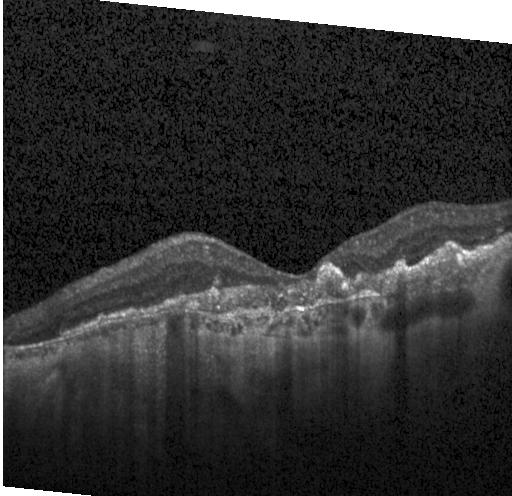
Finding: a choroidal neovascular membrane.